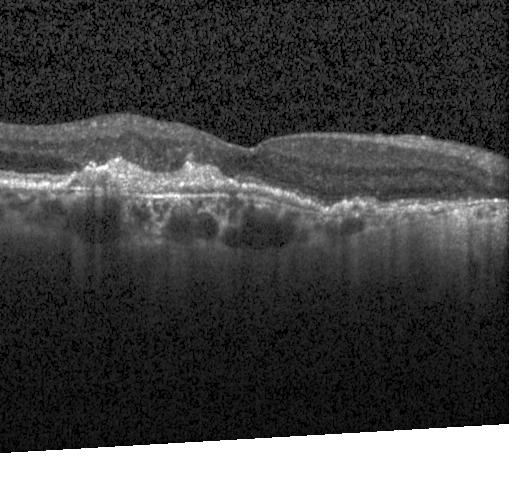

Spectral-domain optical coherence tomography, horizontal scan through the fovea, optical coherence tomography B-scan, acquired on a Heidelberg Spectralis
Finding: a choroidal neovascular membrane.